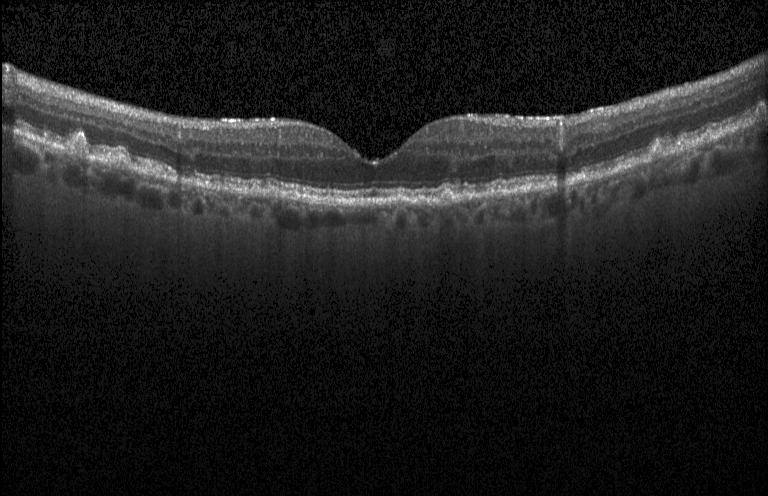

Spectral-domain optical coherence tomography, retinal OCT B-scan
Diagnosis: multiple drusen.